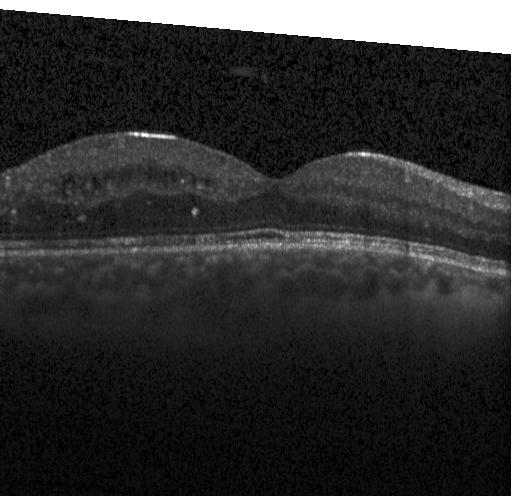

Instrument: Heidelberg Spectralis; OCT B-scan; through the macula; spectral-domain optical coherence tomography
This B-scan demonstrates diabetic macular edema (DME).